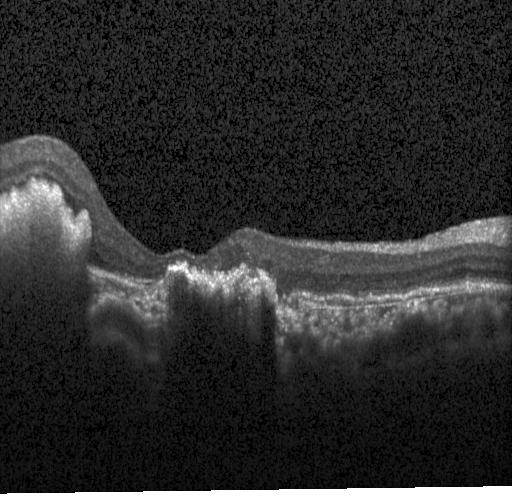
SD-OCT. Macular scan. Instrument: Heidelberg Spectralis. Retinal OCT cross-section. Assessment: a choroidal neovascular membrane.